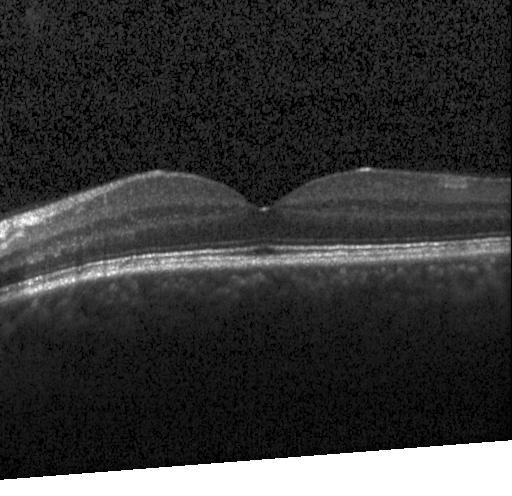
Optical coherence tomography scan. The scan shows no evidence of choroidal neovascularization, diabetic macular edema, or drusen.